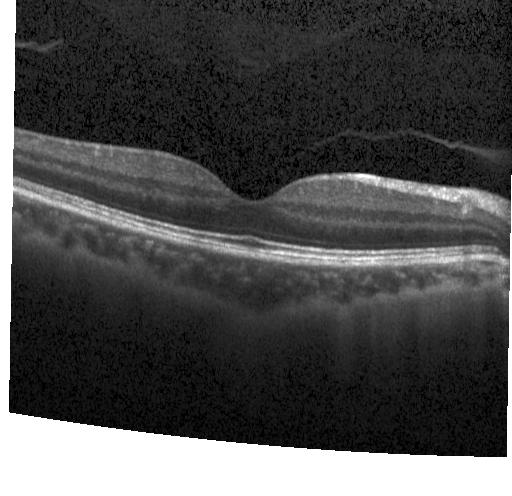 Retinal OCT cross-section showing no choroidal neovascularization, diabetic macular edema, or drusen.